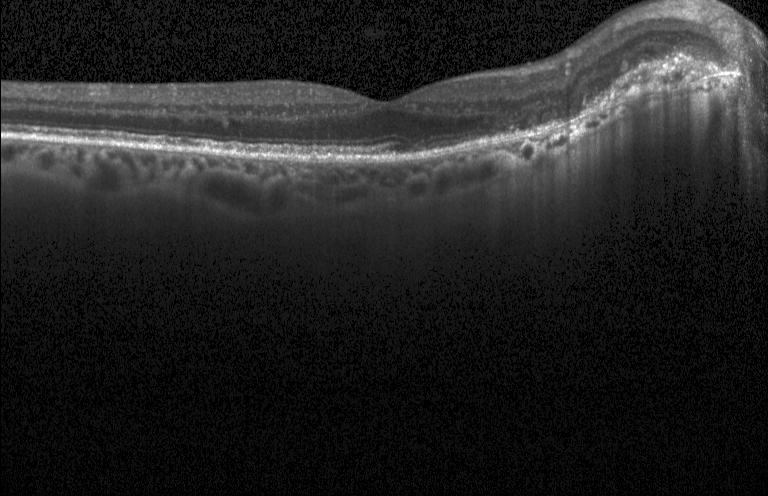 Dx: a choroidal neovascular membrane.